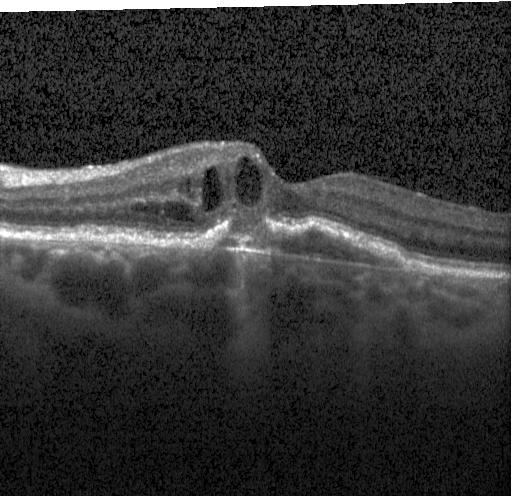 Finding: CNV.